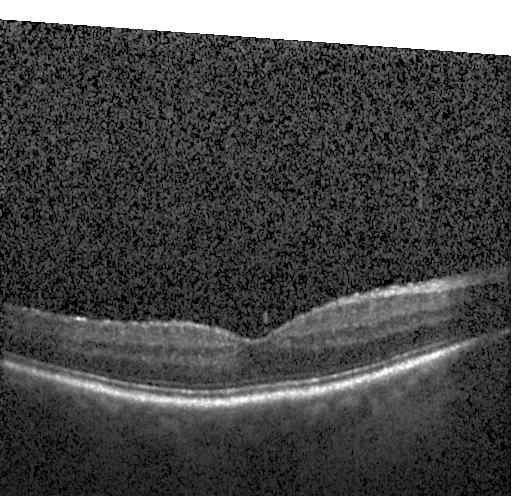

Heidelberg Spectralis OCT system; retinal OCT cross-section.
The scan shows no choroidal neovascularization, no diabetic macular edema, and no drusen.